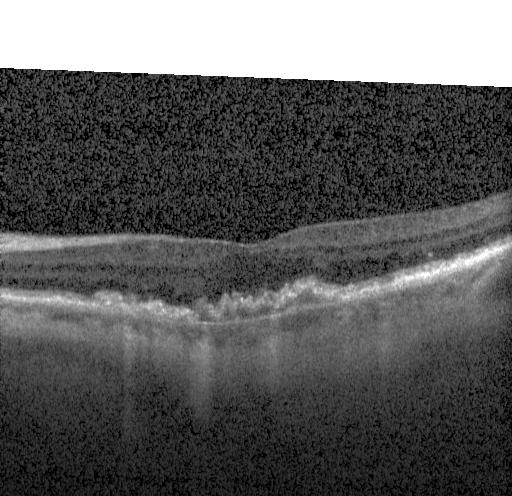
Impression: a choroidal neovascular membrane.